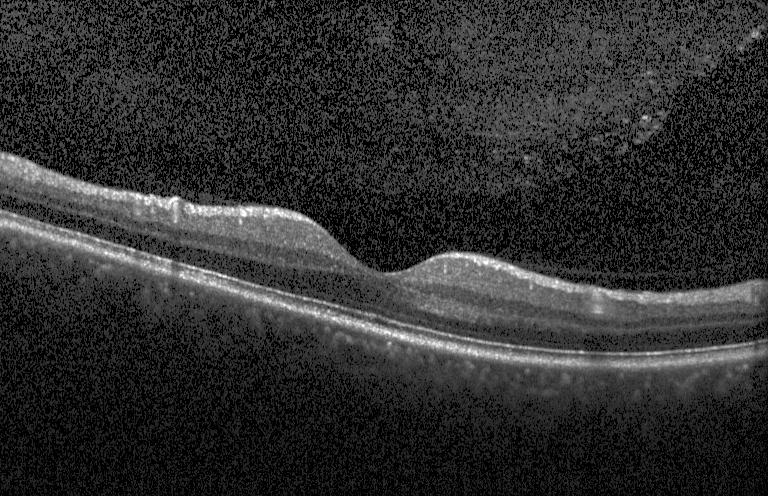 Finding: no CNV, DME, or drusen.